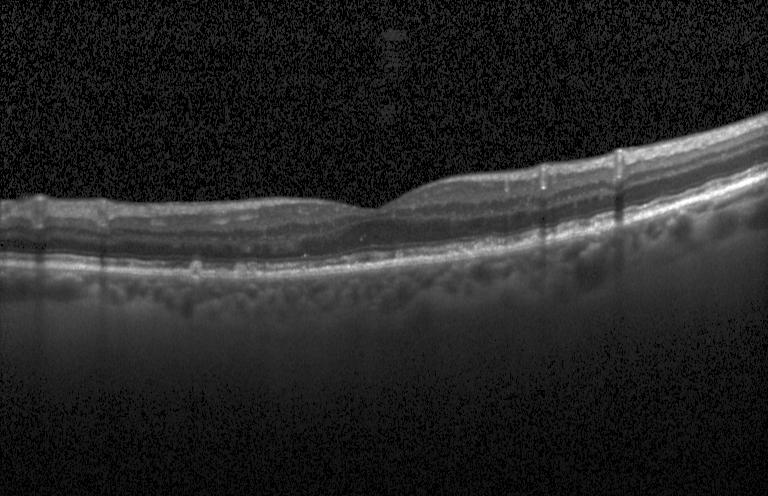

Retinal OCT cross-section; fovea-centered; spectral-domain OCT; Heidelberg Spectralis OCT system — The scan shows multiple drusen.